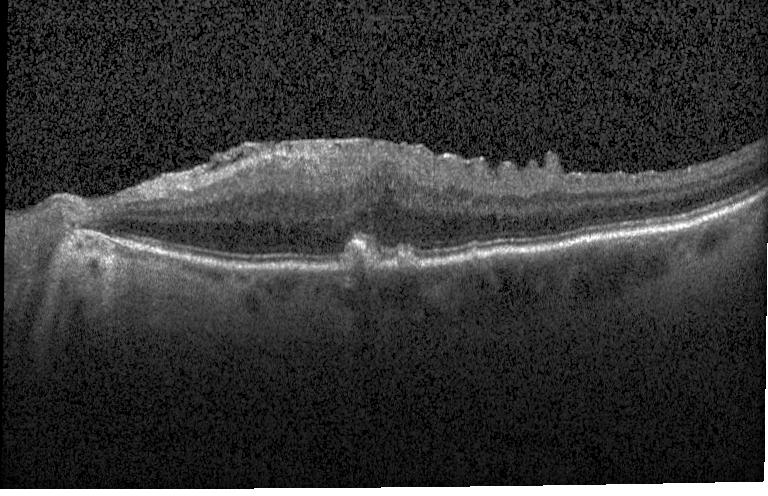

Fovea-centered, Heidelberg Spectralis OCT system, OCT line scan, SD-OCT. Finding: drusen.